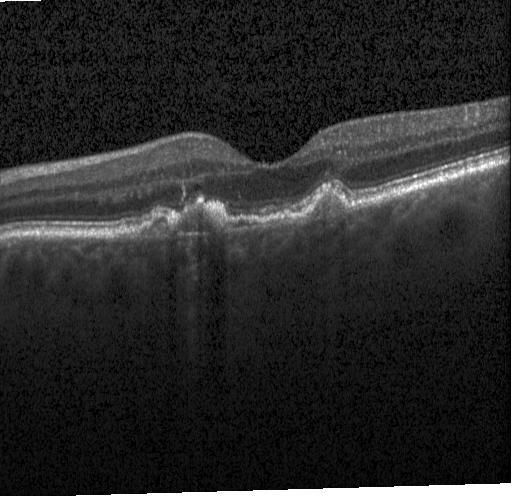
Retinal OCT cross-section. Instrument: Heidelberg Spectralis. SD-OCT. Through the macula
Macular OCT: a choroidal neovascular membrane.